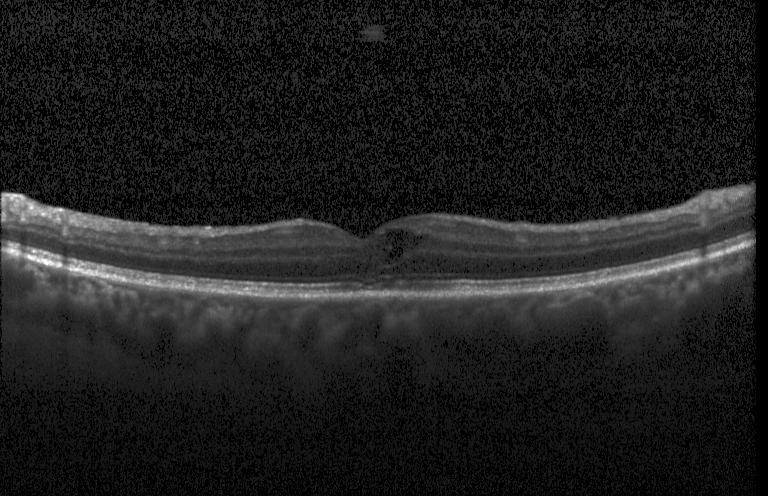
Retinal OCT cross-section. Instrument: Heidelberg Spectralis
Diabetic macular edema (DME).